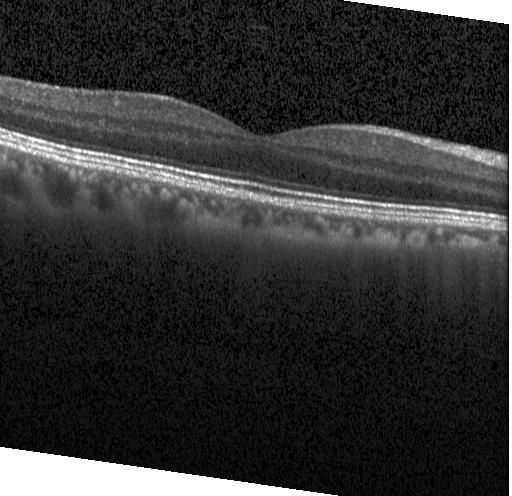 Assessment: no choroidal neovascularization, no diabetic macular edema, and no drusen.